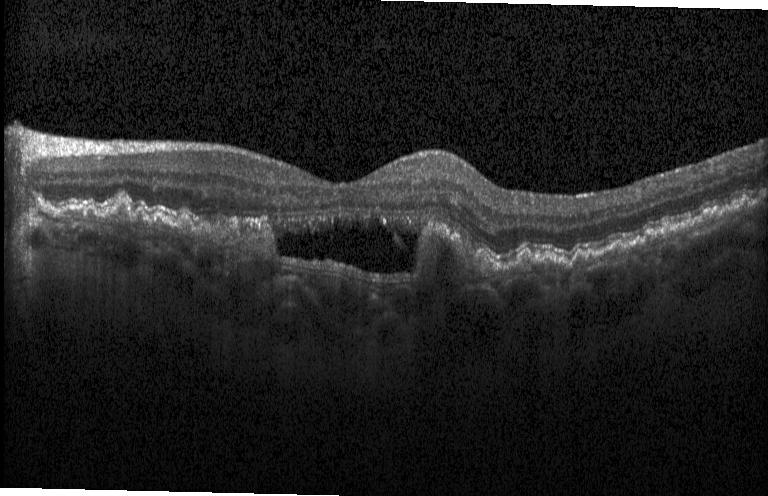

Acquired on a Heidelberg Spectralis, optical coherence tomography B-scan.
This B-scan demonstrates a choroidal neovascular membrane.